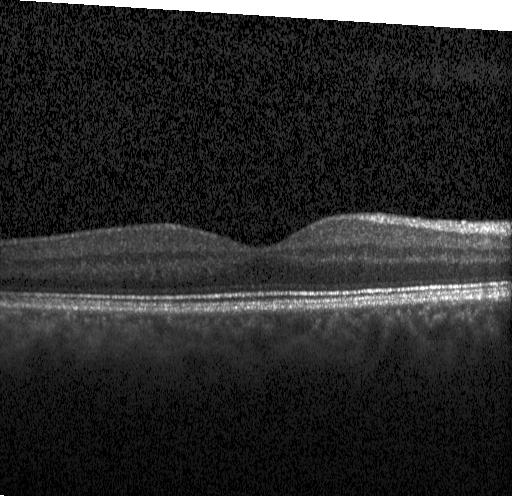 Horizontal scan through the fovea · instrument: Heidelberg Spectralis · OCT B-scan · spectral-domain OCT. Dx: neither choroidal neovascularization, diabetic macular edema, nor drusen.